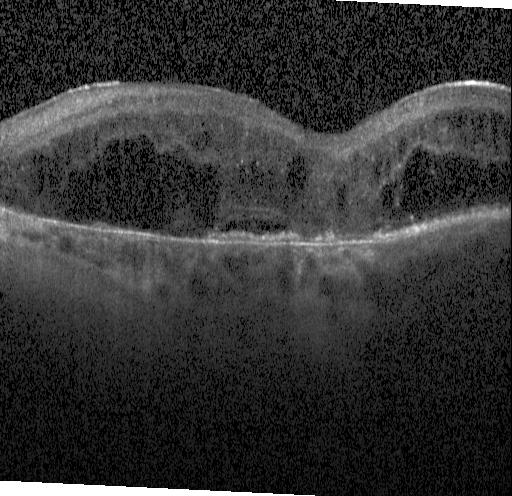 Retinal OCT cross-section, macular scan
Finding: choroidal neovascularization (CNV).